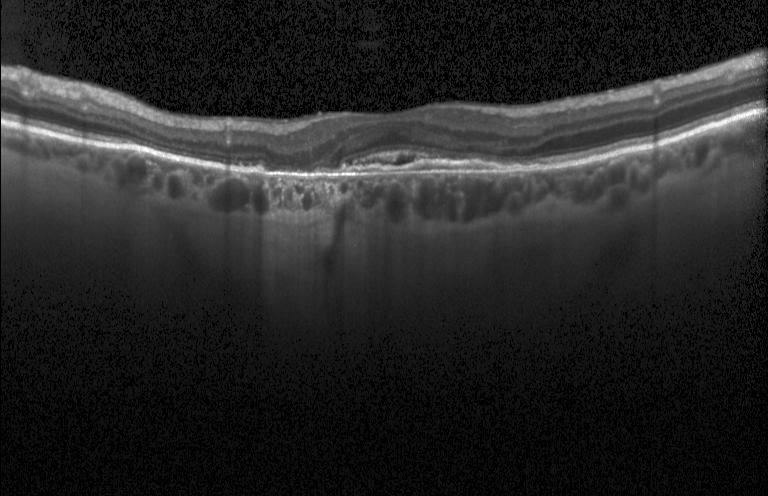

Finding: choroidal neovascularization (CNV).